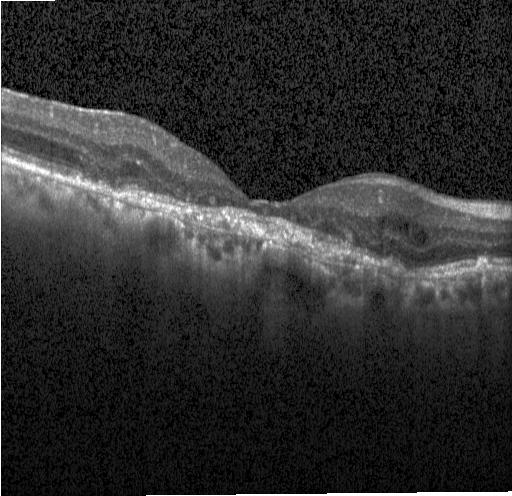
Optical coherence tomography scan. Diagnosis: a choroidal neovascular membrane.